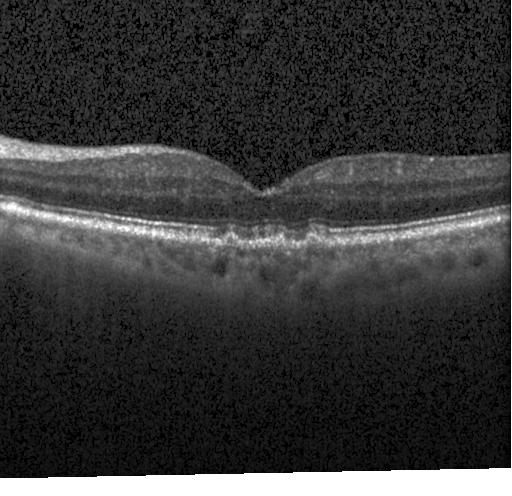

Instrument: Heidelberg Spectralis, centered on the fovea, OCT B-scan, spectral-domain optical coherence tomography.
Dx: sub-RPE drusenoid deposits.